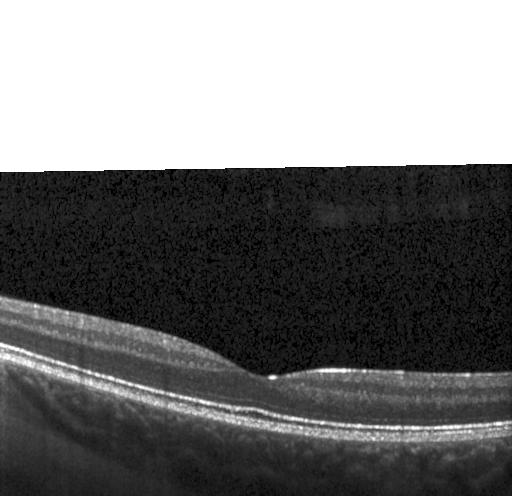
Optical coherence tomography B-scan. Spectral-domain OCT. OCT finding: no choroidal neovascularization, no diabetic macular edema, and no drusen.